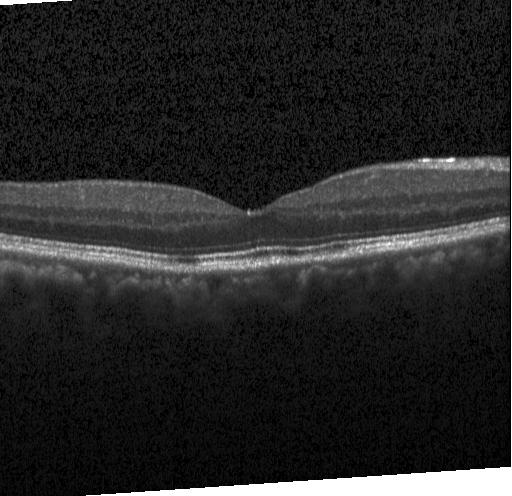

Spectral-domain optical coherence tomography. Retinal OCT B-scan — Diagnosis: neither choroidal neovascularization, diabetic macular edema, nor drusen.